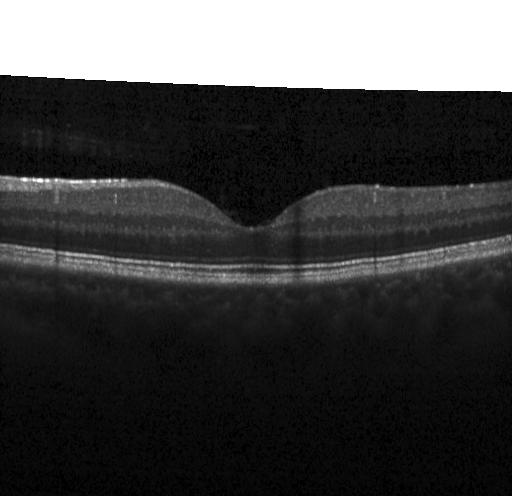

Retinal OCT cross-section. Finding: no evidence of choroidal neovascularization, diabetic macular edema, or drusen.